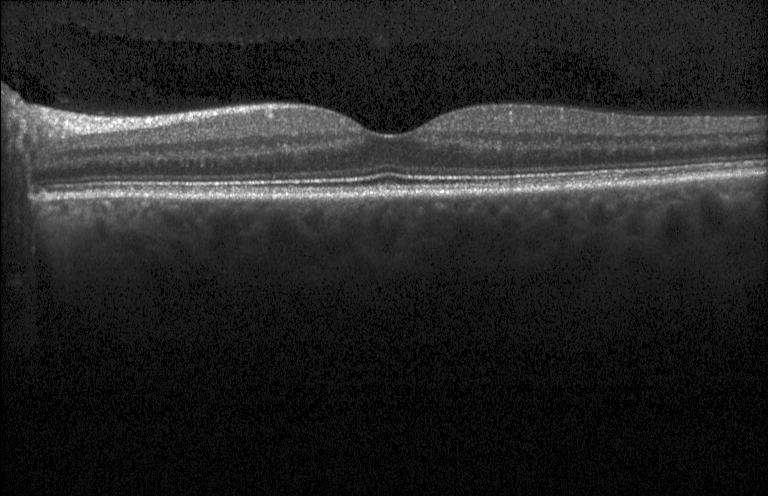
OCT scan showing no CNV, no DME, and no drusen.